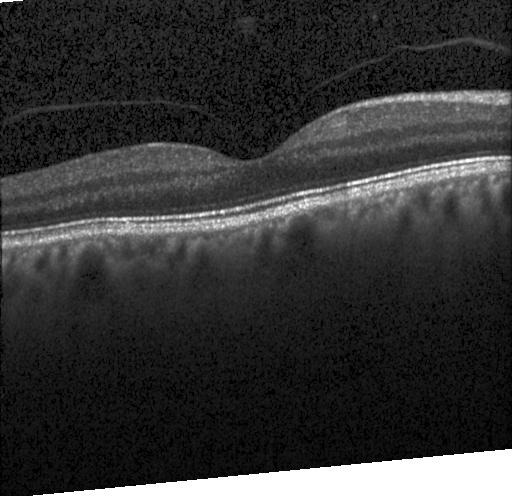 Retinal OCT cross-section. Impression: no CNV, no DME, and no drusen.